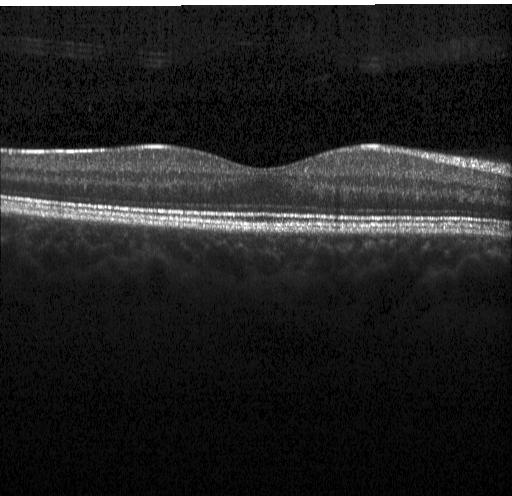 Heidelberg Spectralis, horizontal scan through the fovea, spectral-domain OCT, retinal OCT B-scan — Dx: neither choroidal neovascularization, diabetic macular edema, nor drusen.